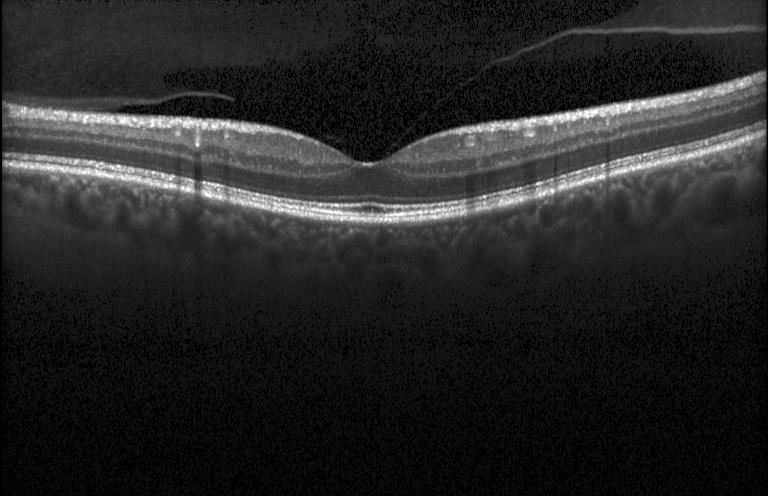
Retinal OCT cross-section.
Finding: no CNV, no DME, and no drusen.